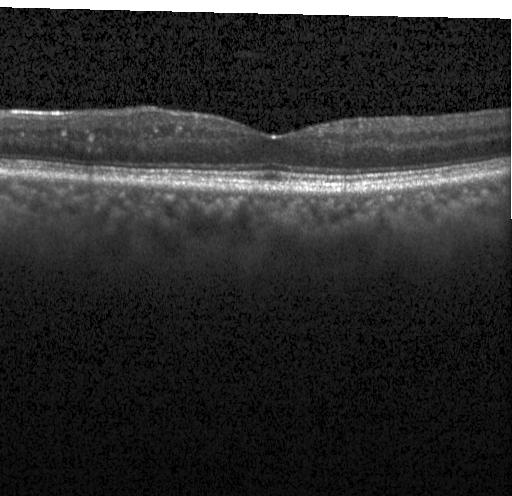 Optical coherence tomography B-scan.
No CNV, no DME, and no drusen.